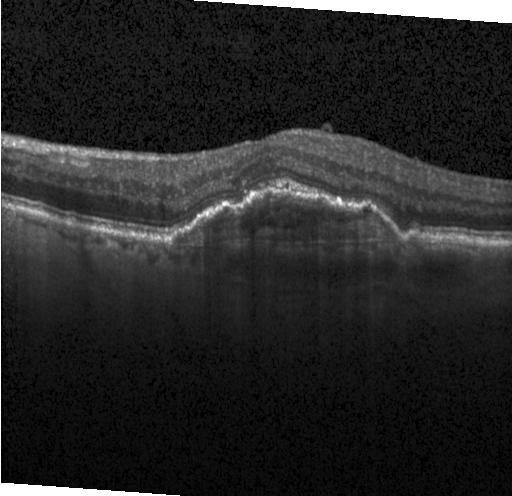 OCT line scan — This B-scan demonstrates choroidal neovascularization.